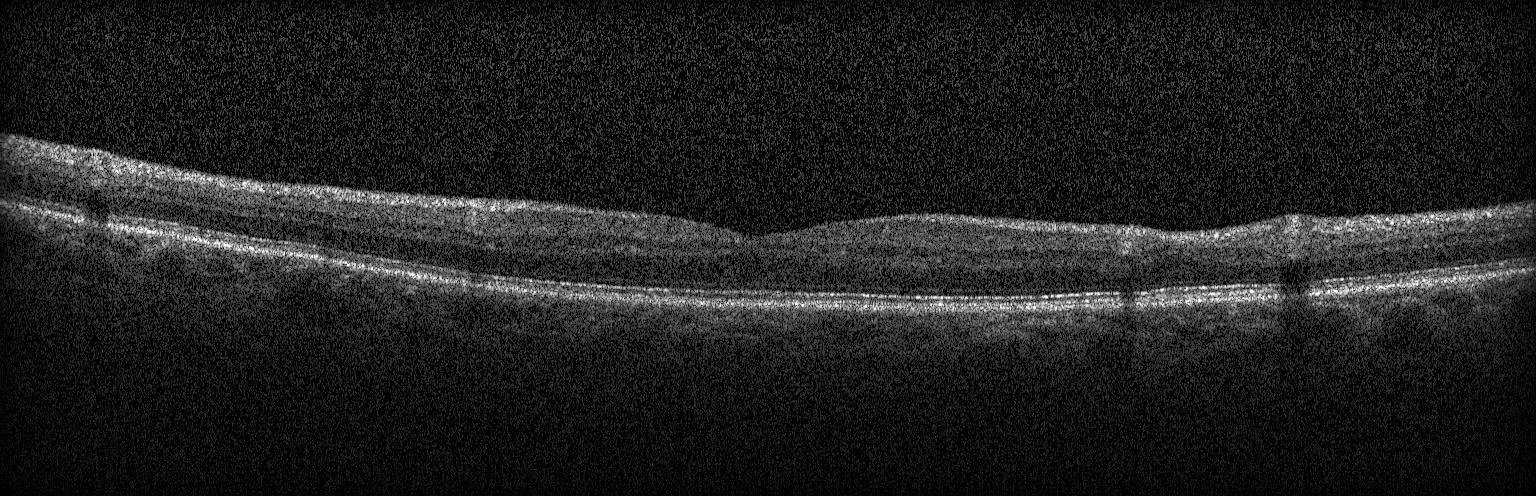

Assessment: no CNV, DME, or drusen.